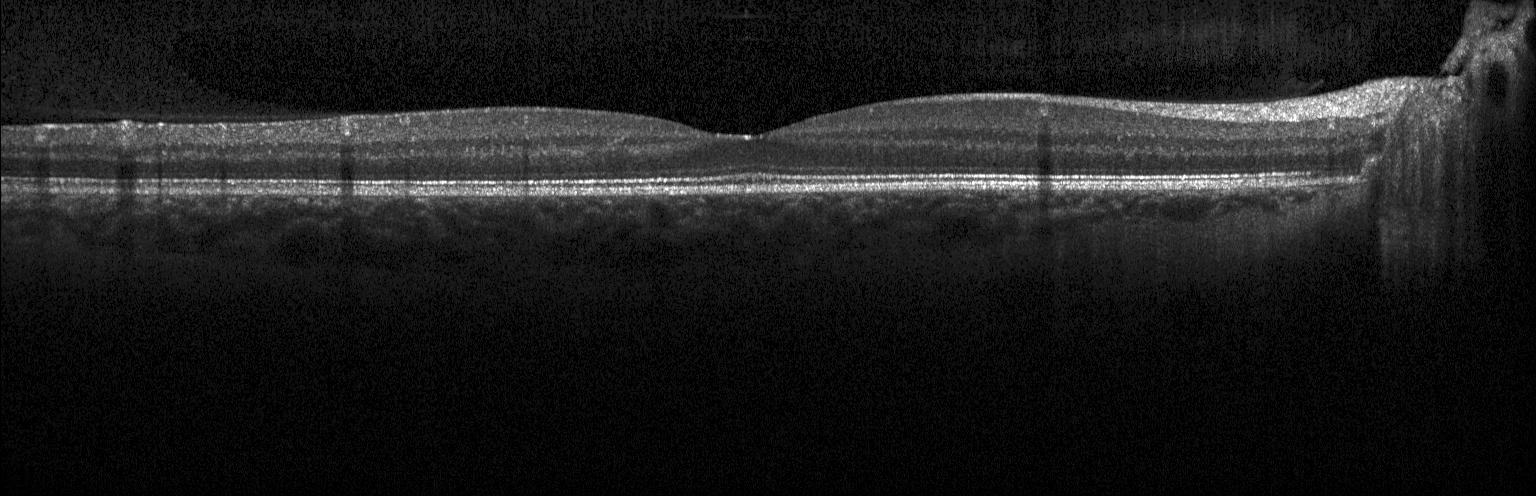

Diagnosis: neither choroidal neovascularization, diabetic macular edema, nor drusen.